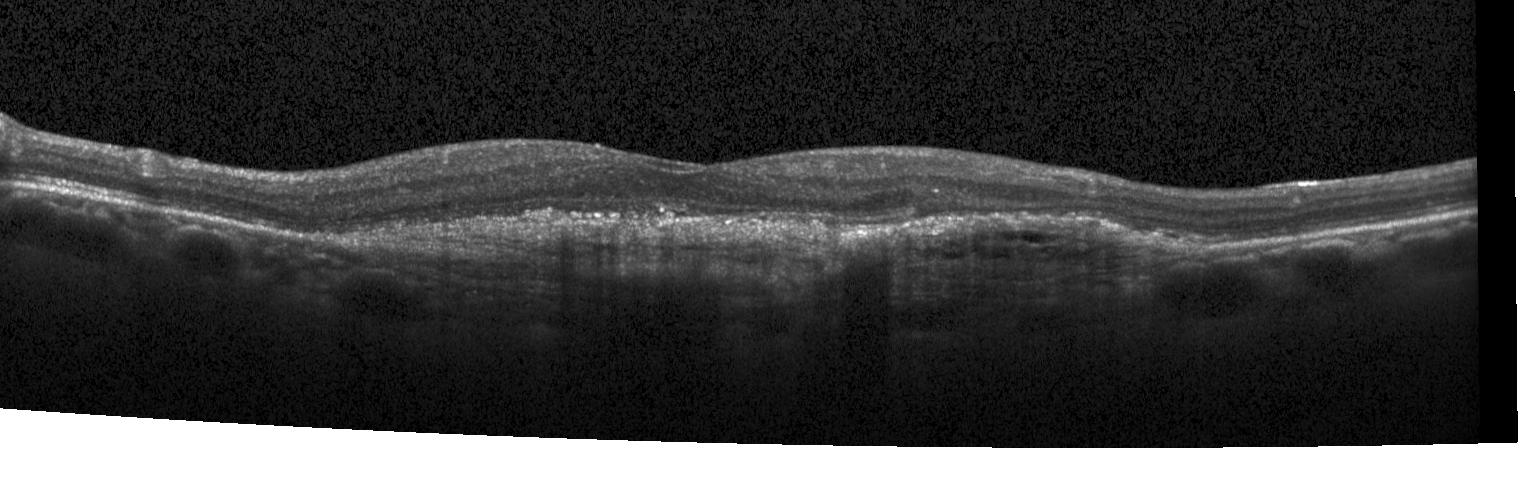 Instrument: Heidelberg Spectralis. Centered on the fovea. Optical coherence tomography scan. SD-OCT
Impression: choroidal neovascularization.